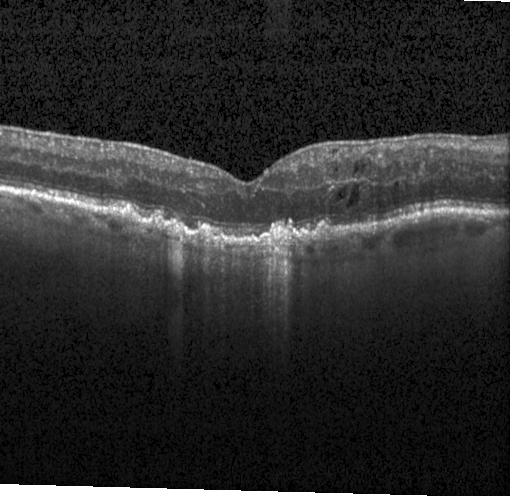 Heidelberg Spectralis, optical coherence tomography scan, SD-OCT.
Diagnosis: a choroidal neovascular membrane.